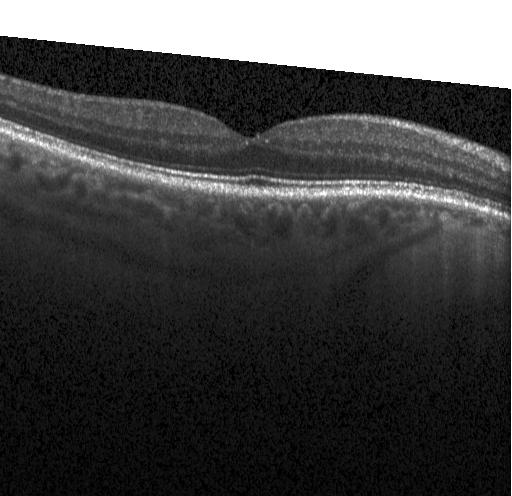
Retinal OCT cross-section · spectral-domain optical coherence tomography
Impression: neither choroidal neovascularization, diabetic macular edema, nor drusen.